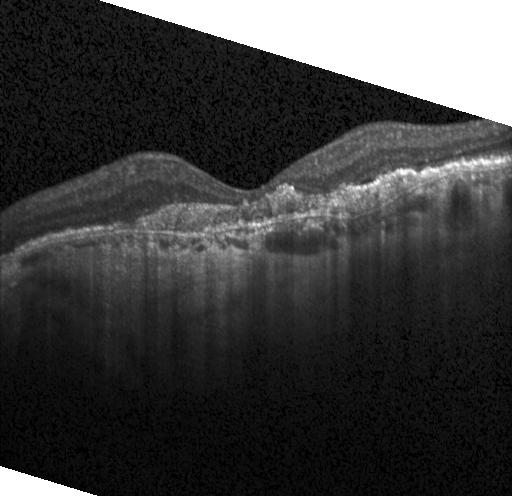

Instrument: Heidelberg Spectralis · optical coherence tomography scan · through the macula · SD-OCT
Impression: a choroidal neovascular membrane.